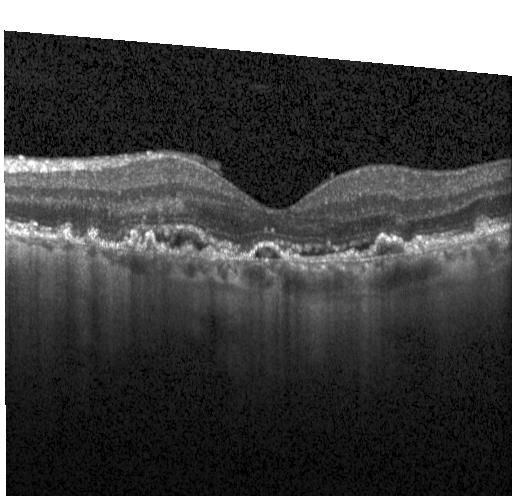
Impression: choroidal neovascularization (CNV).